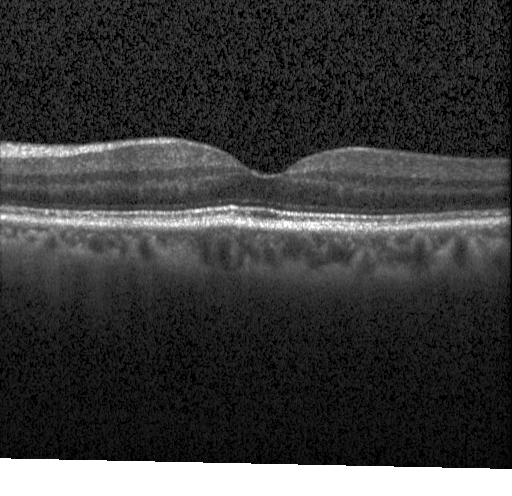

OCT B-scan. Fovea-centered. Spectral-domain OCT. Impression: no choroidal neovascularization, diabetic macular edema, or drusen.